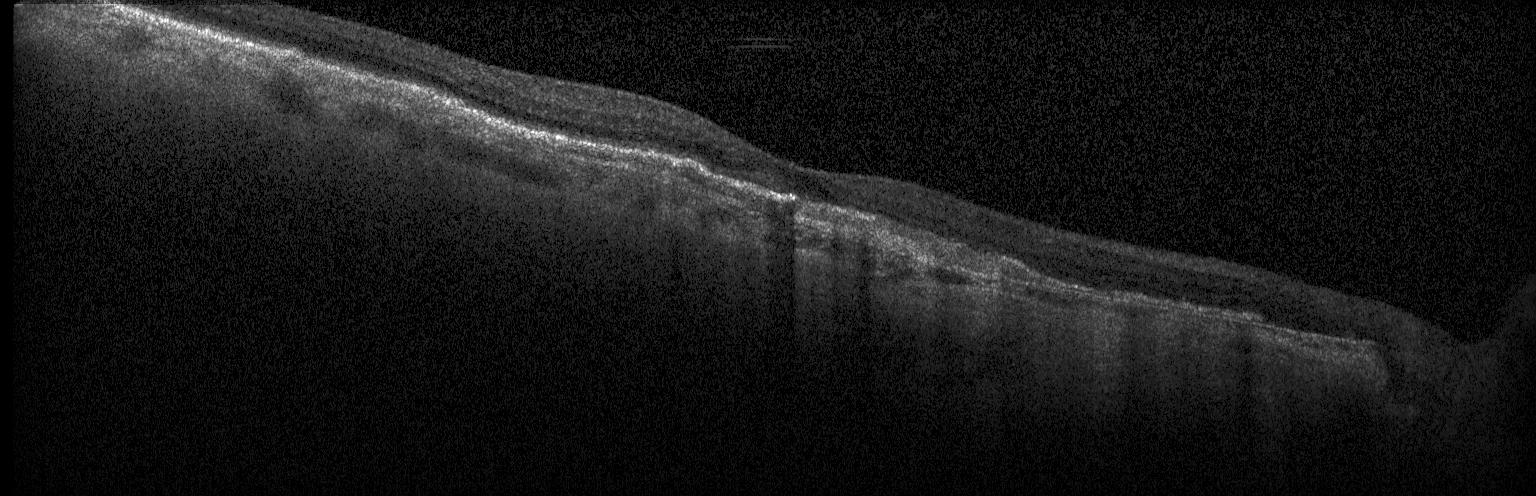
Spectral-domain OCT; optical coherence tomography B-scan; Heidelberg Spectralis OCT system; macular scan — Finding: a choroidal neovascular membrane.